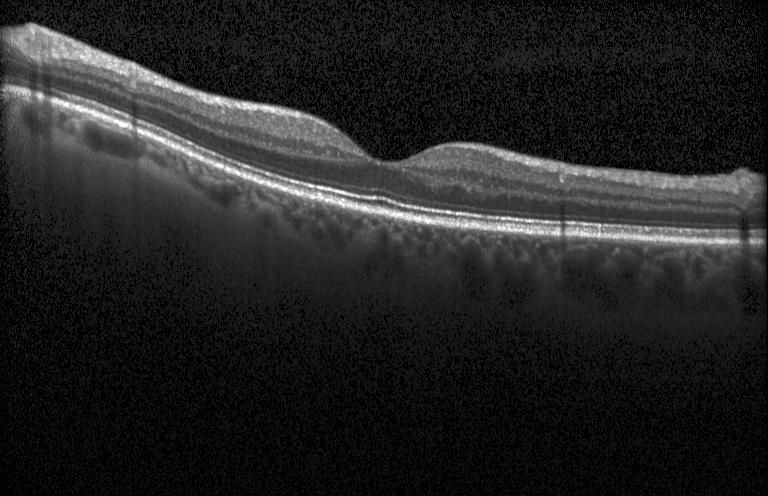
Retinal OCT B-scan — The scan shows no choroidal neovascularization, no diabetic macular edema, and no drusen.